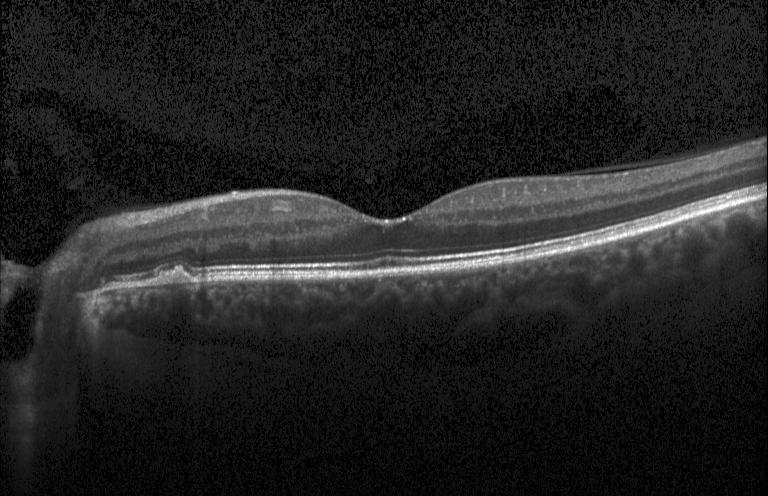
SD-OCT · OCT line scan — Assessment: drusen.